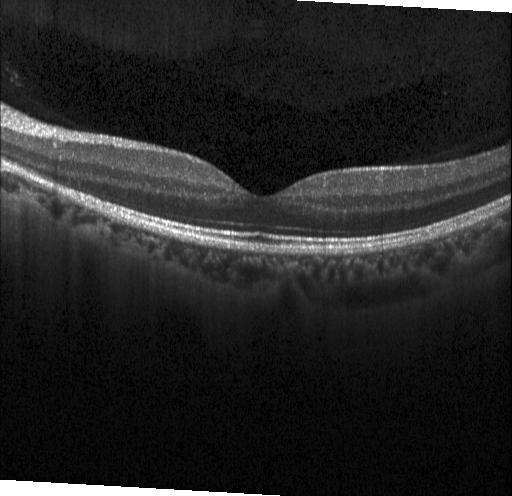
Centered on the fovea. SD-OCT. Retinal OCT cross-section. Heidelberg Spectralis OCT system. Assessment: no choroidal neovascularization, no diabetic macular edema, and no drusen.